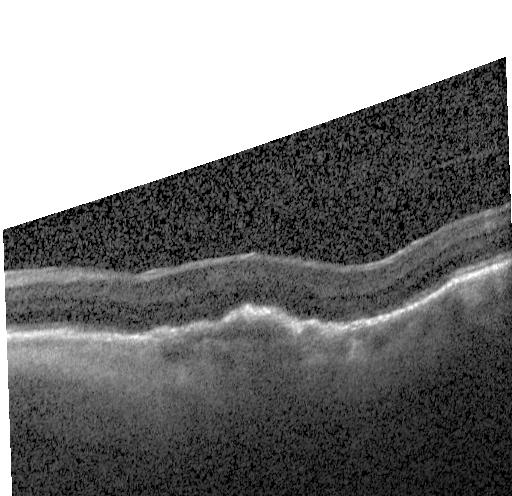
Spectral-domain optical coherence tomography · Heidelberg Spectralis · OCT line scan · through the macula
Finding: a choroidal neovascular membrane.